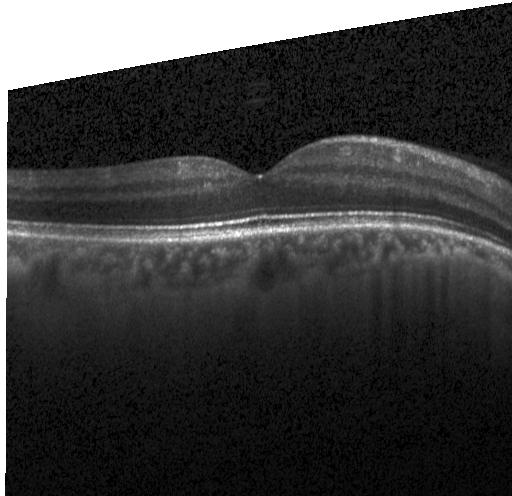 Macular OCT demonstrating neither choroidal neovascularization, diabetic macular edema, nor drusen.